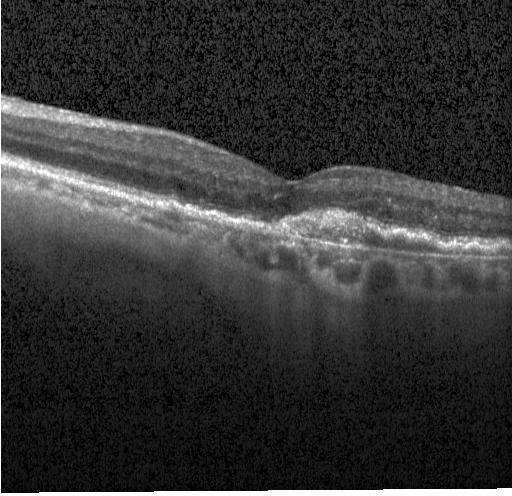
OCT line scan
Impression: choroidal neovascularization (CNV).